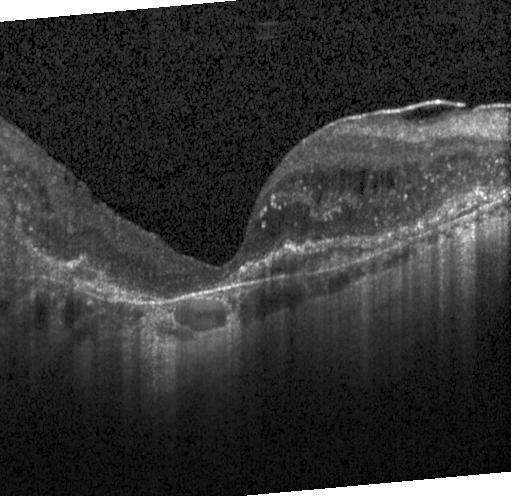 OCT B-scan · macular scan.
CNV.